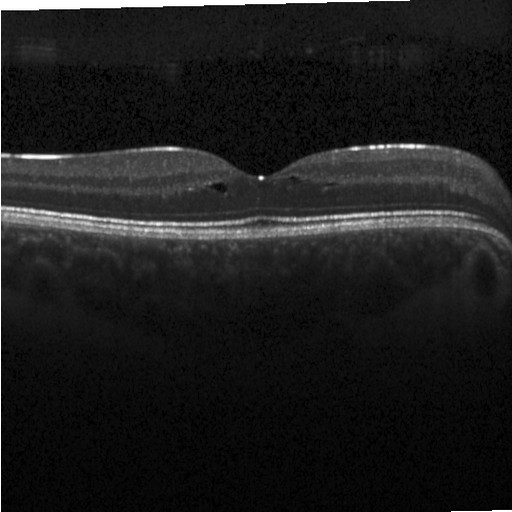
Optical coherence tomography scan; Heidelberg Spectralis; spectral-domain optical coherence tomography — Dx: diabetic macular edema.